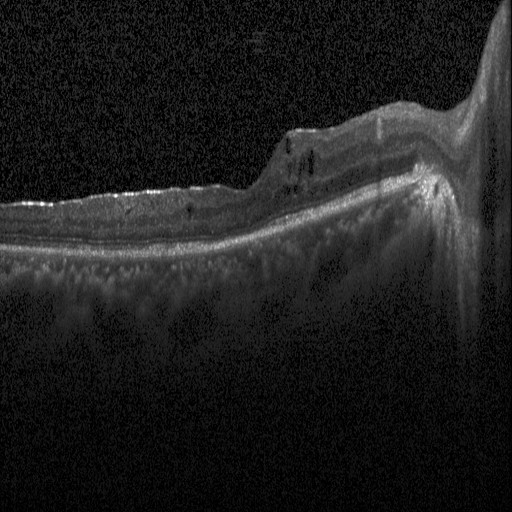
The scan shows diabetic macular edema (DME).